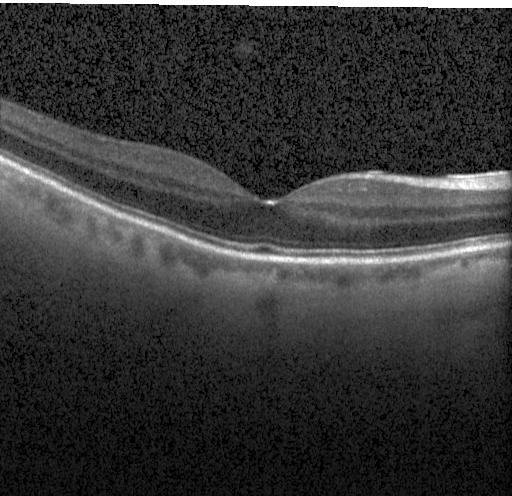 Impression: no evidence of choroidal neovascularization, diabetic macular edema, or drusen.